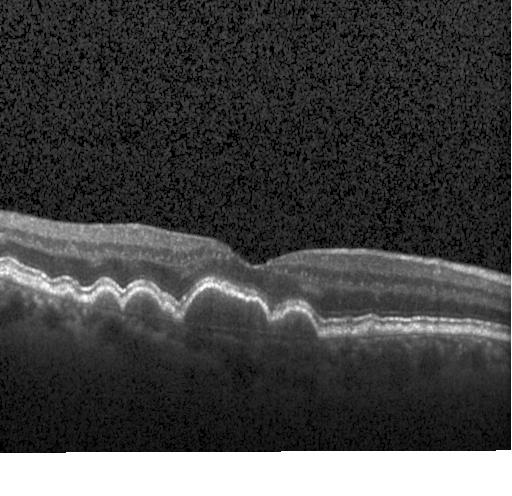
Centered on the fovea. Heidelberg Spectralis OCT system. SD-OCT. Optical coherence tomography scan
Diagnosis: multiple drusen.